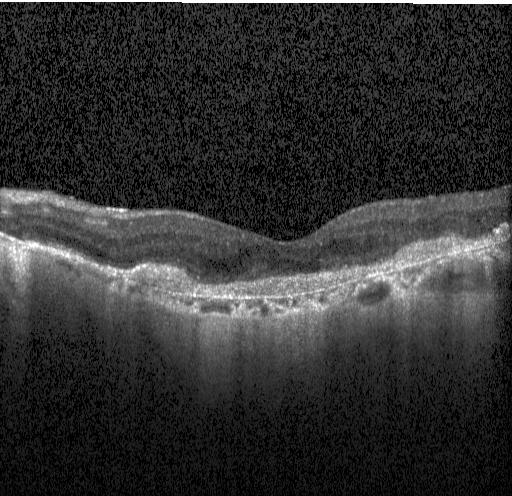
OCT B-scan.
Assessment: CNV.